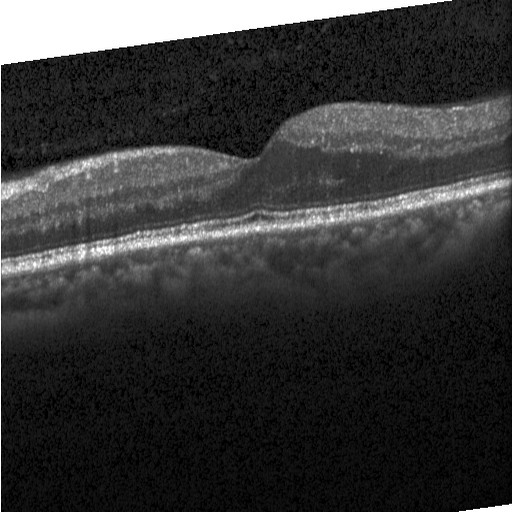
This B-scan demonstrates diabetic macular edema.